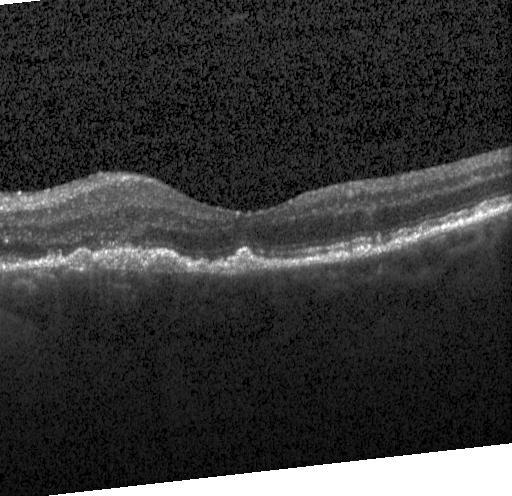 Optical coherence tomography B-scan. Instrument: Heidelberg Spectralis.
A choroidal neovascular membrane.